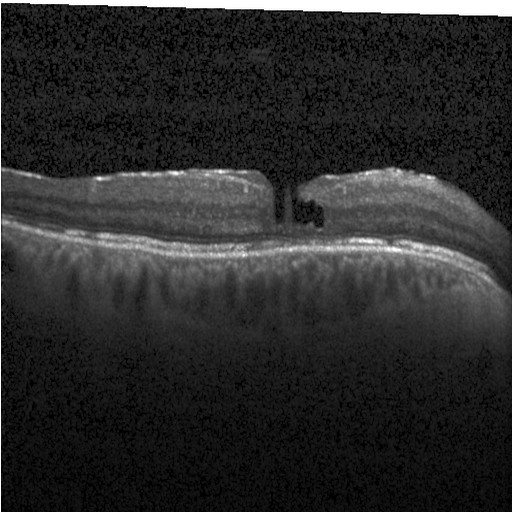 Diagnosis: diabetic macular edema (DME).